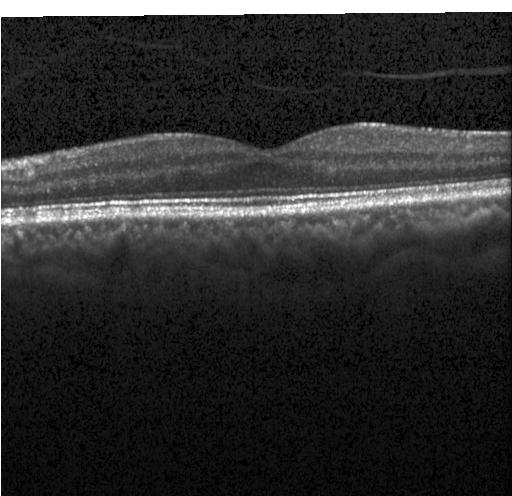
Retinal OCT B-scan.
This B-scan demonstrates neither choroidal neovascularization, diabetic macular edema, nor drusen.